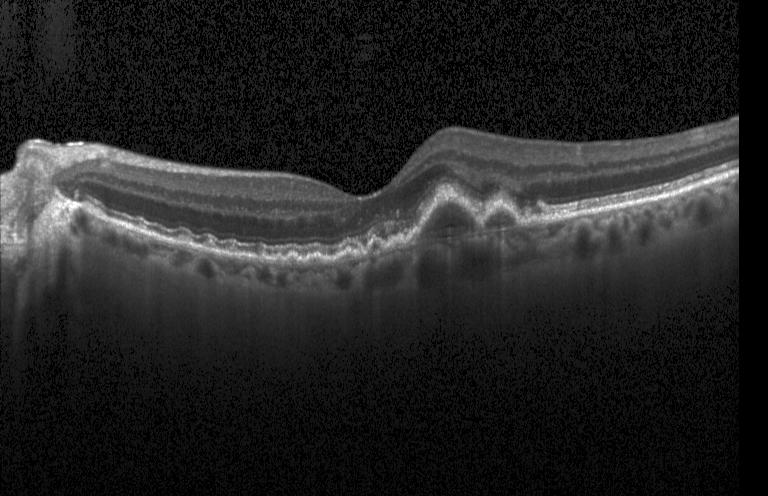

Retinal OCT B-scan; Heidelberg Spectralis OCT system; spectral-domain OCT — The scan shows drusen.